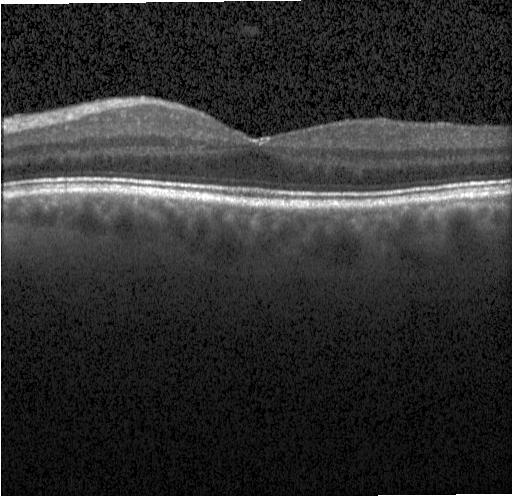

Optical coherence tomography scan. Macular scan. Heidelberg Spectralis OCT system. Spectral-domain OCT — Diagnosis: no CNV, no DME, and no drusen.